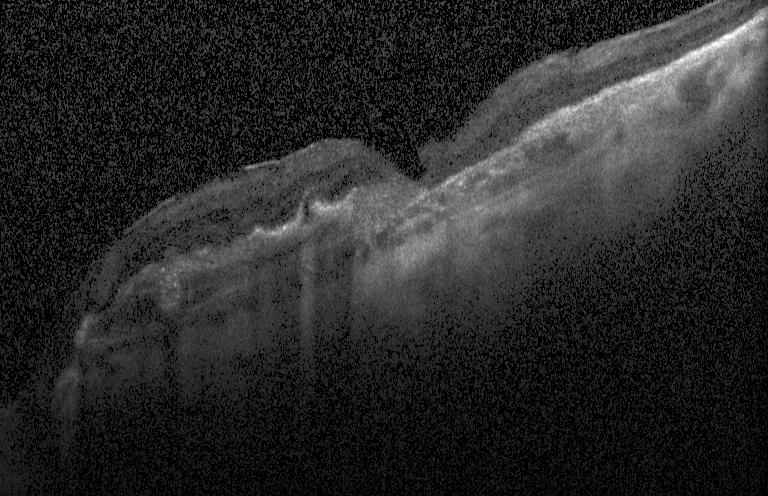 Diagnosis: CNV.